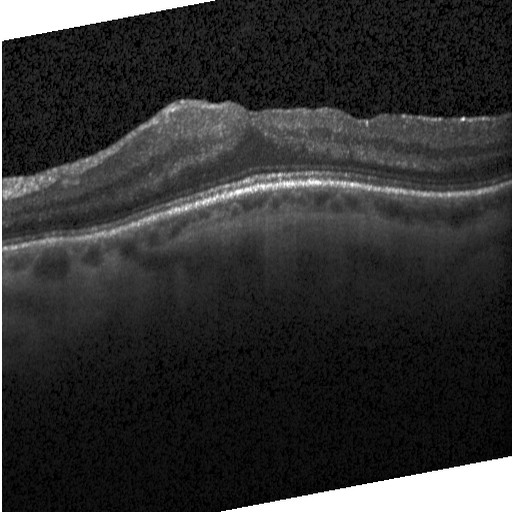

Retinal OCT cross-section
This B-scan demonstrates DME.